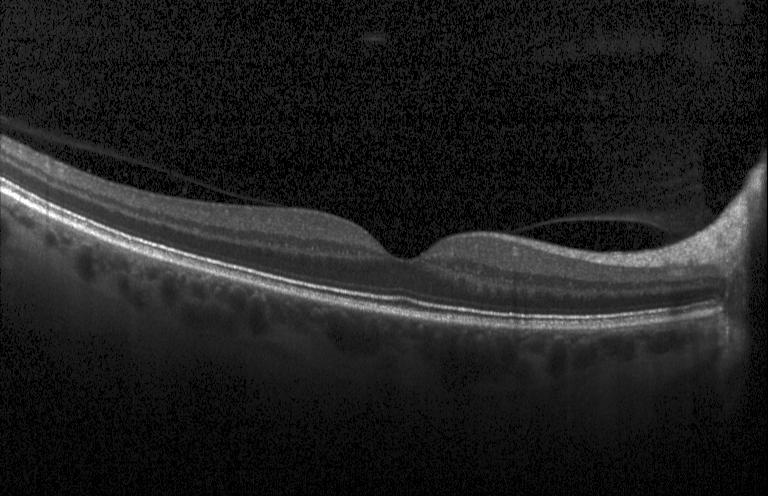

Dx: no evidence of CNV, DME, or drusen.